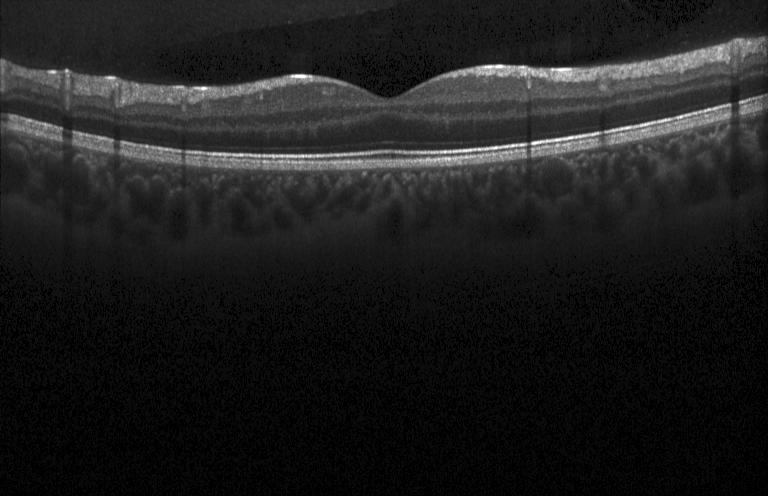
Macular scan. Heidelberg Spectralis OCT system. SD-OCT. OCT line scan. The scan shows no choroidal neovascularization, no diabetic macular edema, and no drusen.